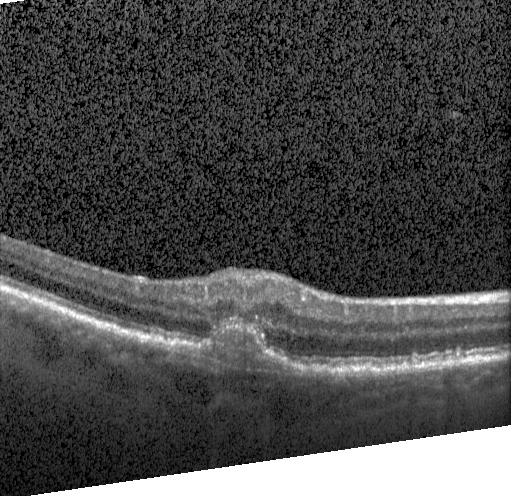

Optical coherence tomography scan · macular scan · spectral-domain OCT.
Finding: choroidal neovascularization.